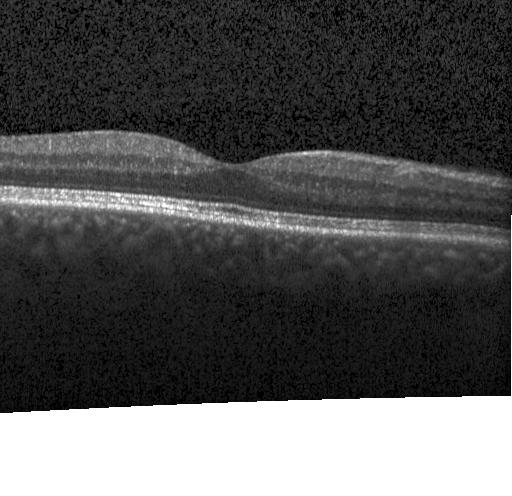 SD-OCT, fovea-centered, OCT line scan, Heidelberg Spectralis.
Diagnosis: no CNV, DME, or drusen.